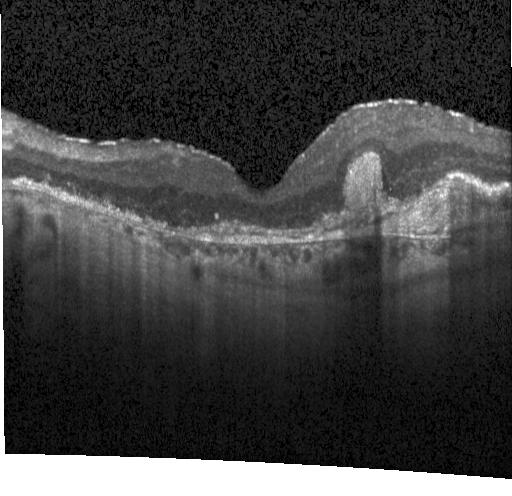 OCT B-scan. Heidelberg Spectralis. A choroidal neovascular membrane.